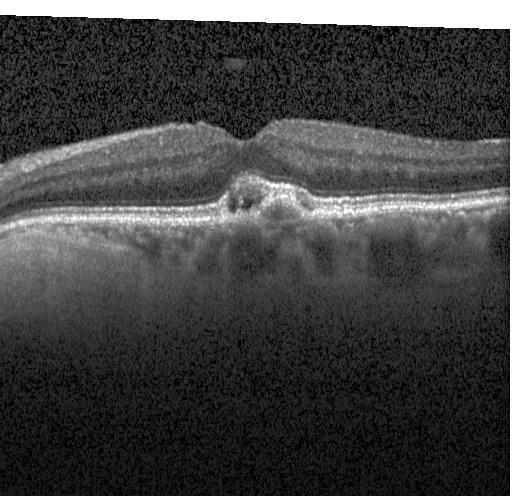
Retinal OCT cross-section showing choroidal neovascularization.